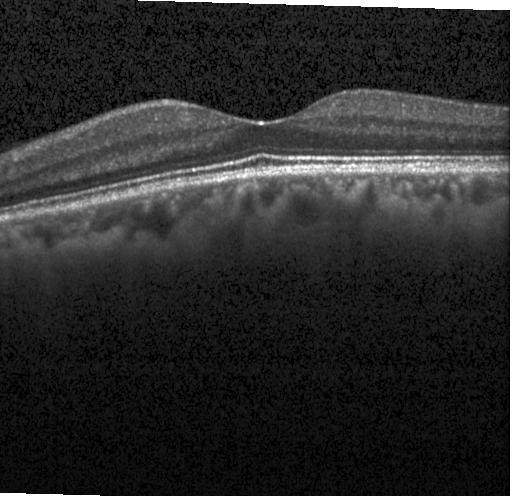 OCT finding: no CNV, DME, or drusen.